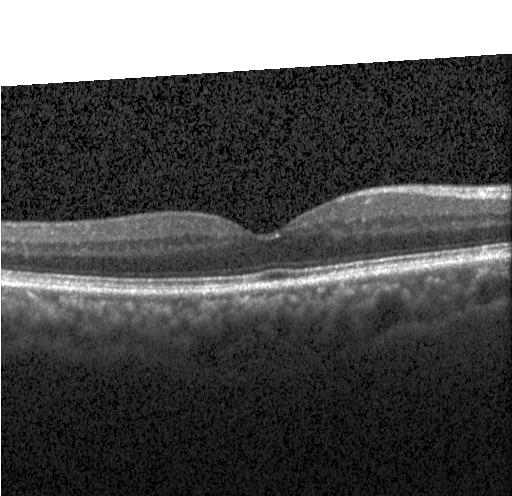

Retinal OCT B-scan — The scan shows no choroidal neovascularization, diabetic macular edema, or drusen.